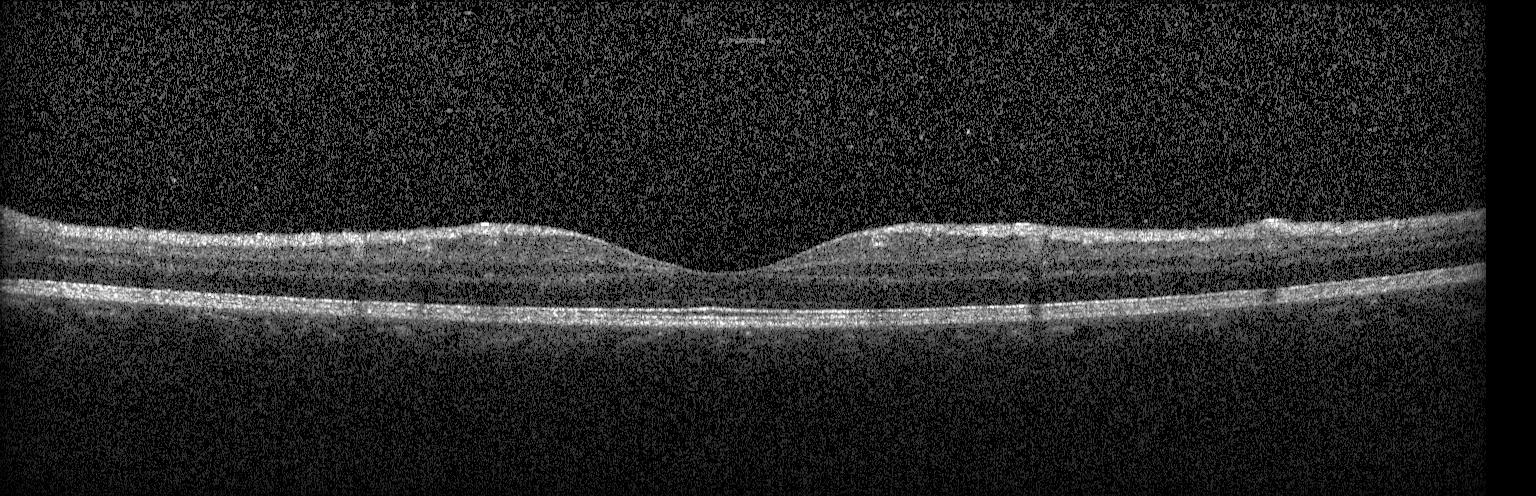

Assessment: no evidence of choroidal neovascularization, diabetic macular edema, or drusen.